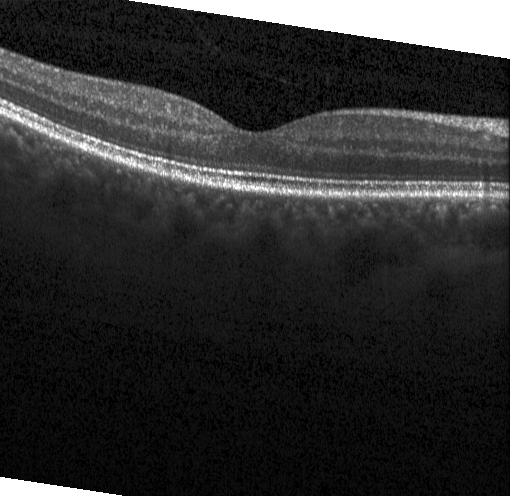 OCT scan showing neither choroidal neovascularization, diabetic macular edema, nor drusen.